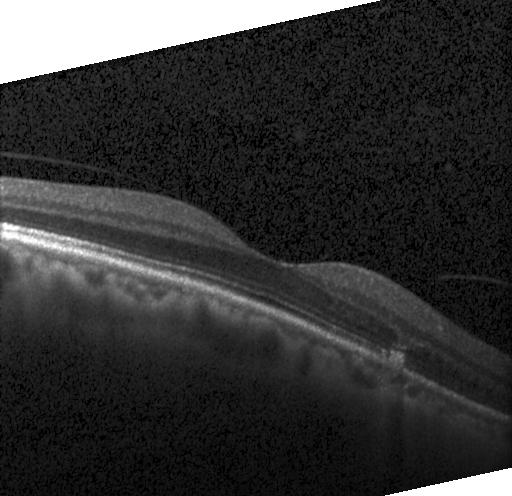
Macular scan · Heidelberg Spectralis · optical coherence tomography B-scan · SD-OCT. This B-scan demonstrates no choroidal neovascularization, no diabetic macular edema, and no drusen.